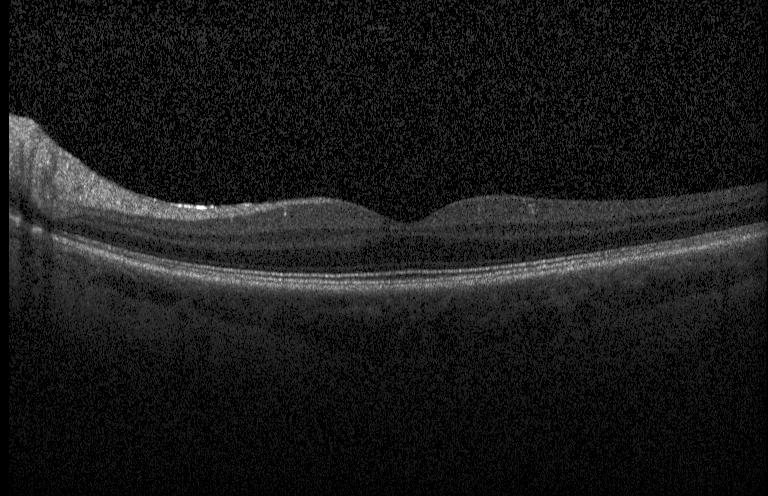

Dx: no CNV, no DME, and no drusen.